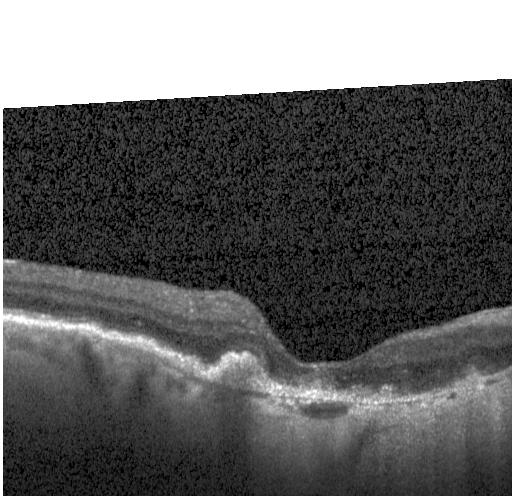 OCT scan showing CNV.